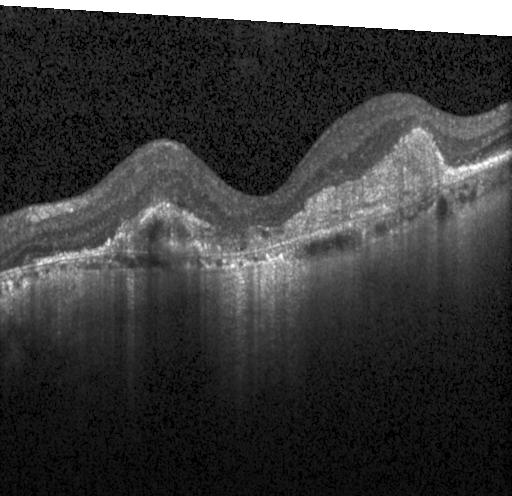
Finding: choroidal neovascularization.